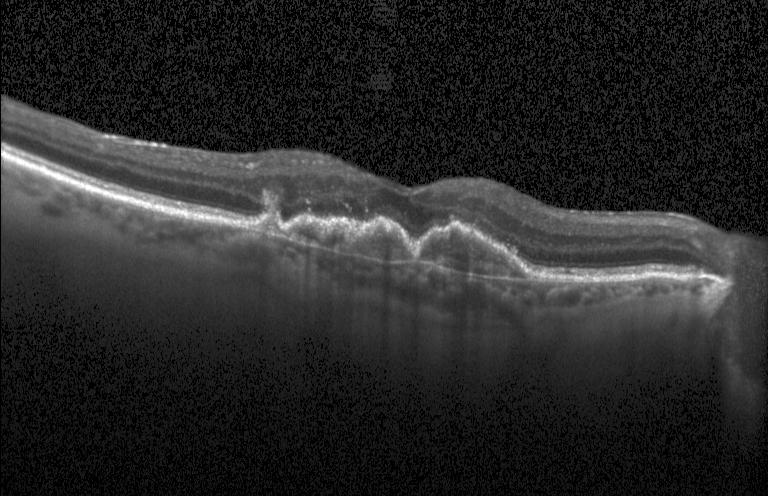

OCT line scan. Spectral-domain optical coherence tomography
Finding: CNV.